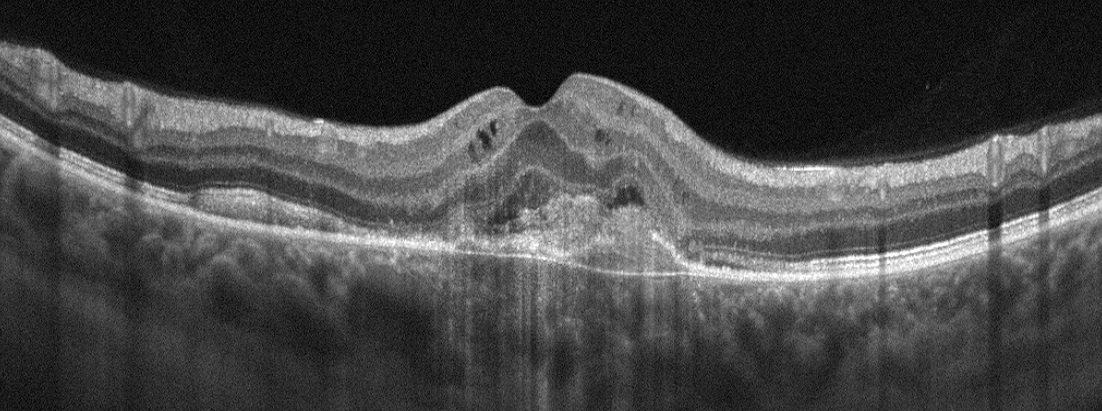

Retinal OCT cross-section showing age-related macular degeneration.